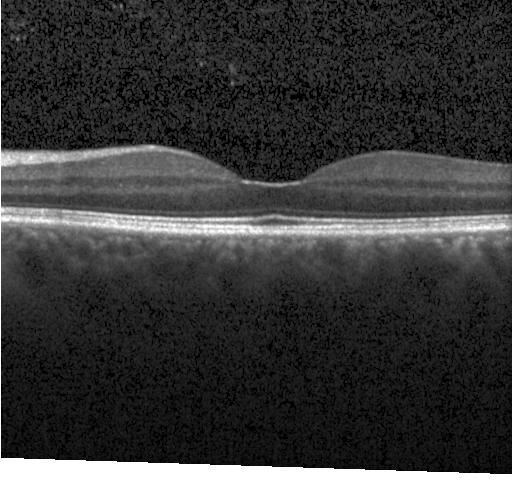
Instrument: Heidelberg Spectralis · optical coherence tomography B-scan — Impression: no choroidal neovascularization, no diabetic macular edema, and no drusen.